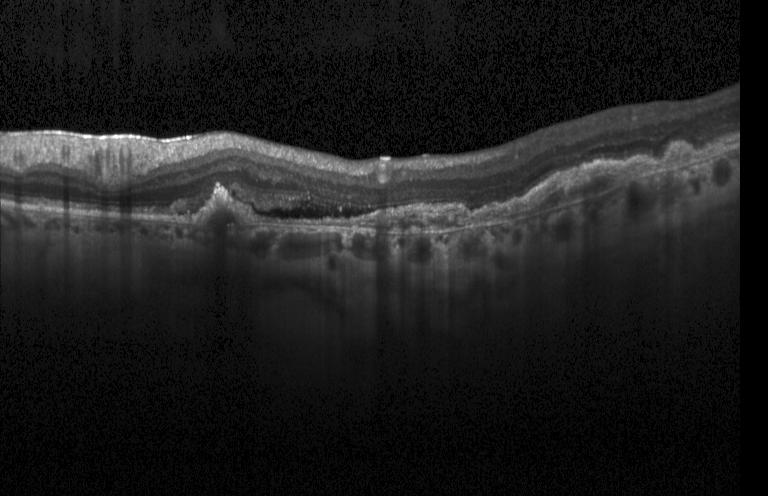 OCT B-scan. The scan shows a choroidal neovascular membrane.